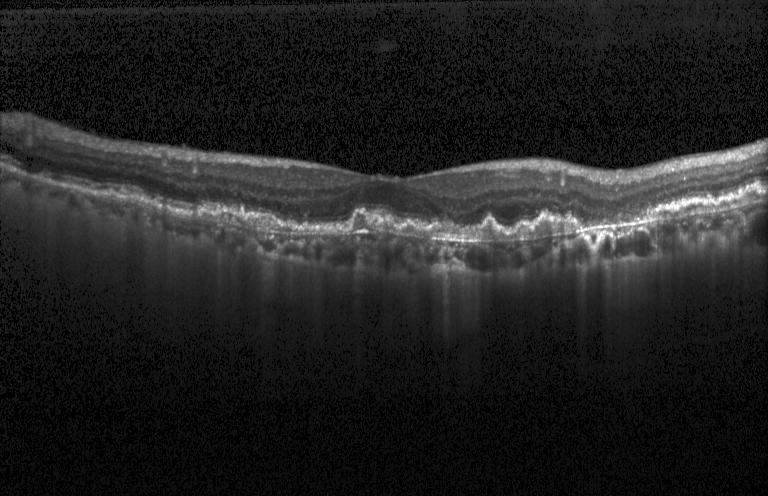

Optical coherence tomography scan.
A choroidal neovascular membrane.